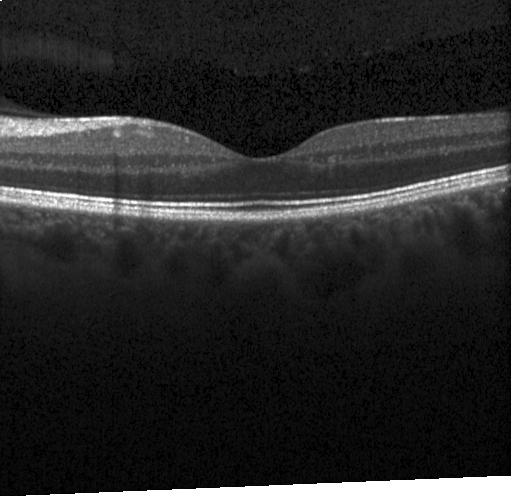

OCT line scan. Fovea-centered. Heidelberg Spectralis. Spectral-domain OCT
Diagnosis: no CNV, DME, or drusen.